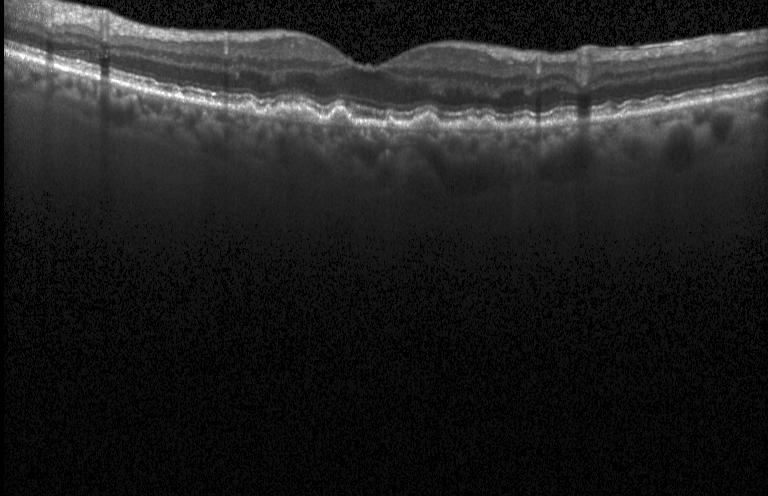 Heidelberg Spectralis. OCT B-scan. Macular scan. Spectral-domain OCT — Finding: drusen.